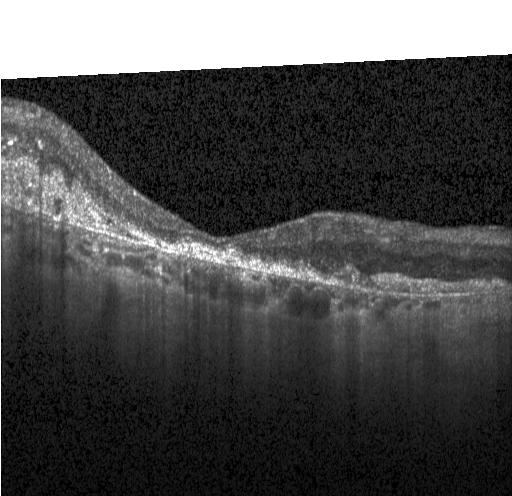

Acquired on a Heidelberg Spectralis. Optical coherence tomography B-scan — Impression: a choroidal neovascular membrane.